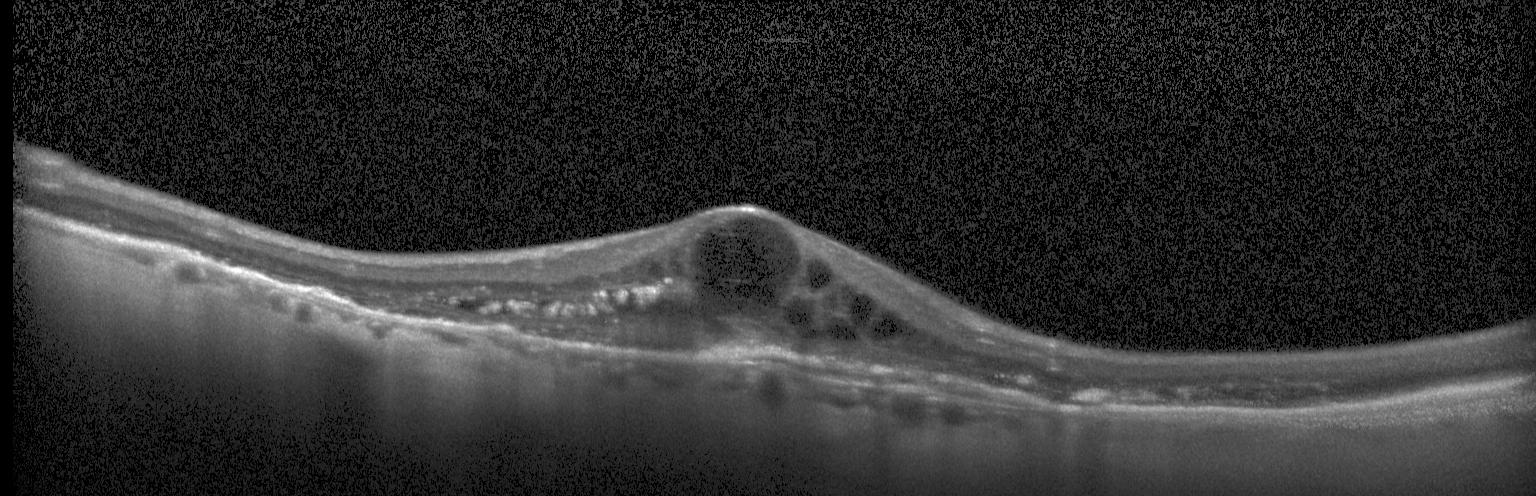 Dx: a choroidal neovascular membrane.